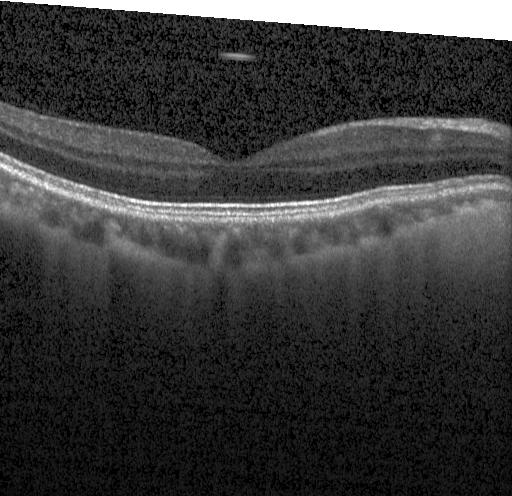
Instrument: Heidelberg Spectralis. OCT line scan. SD-OCT. Macular scan
This B-scan demonstrates no choroidal neovascularization, no diabetic macular edema, and no drusen.